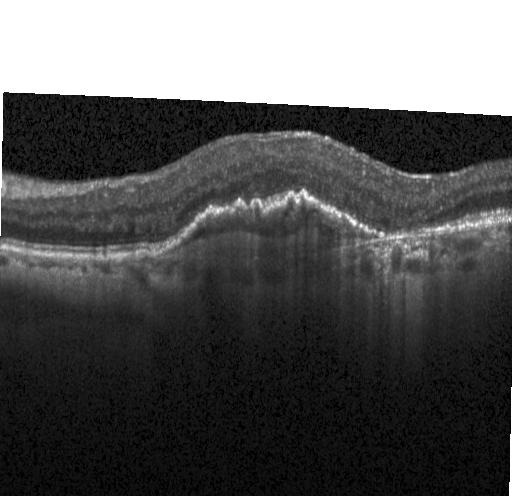 Macular OCT demonstrating a choroidal neovascular membrane.